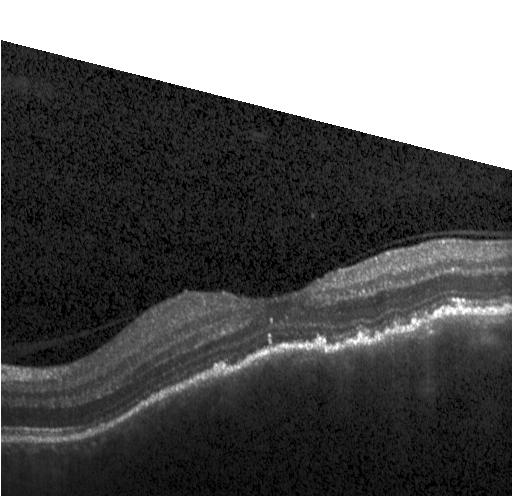 OCT finding: sub-RPE drusenoid deposits.